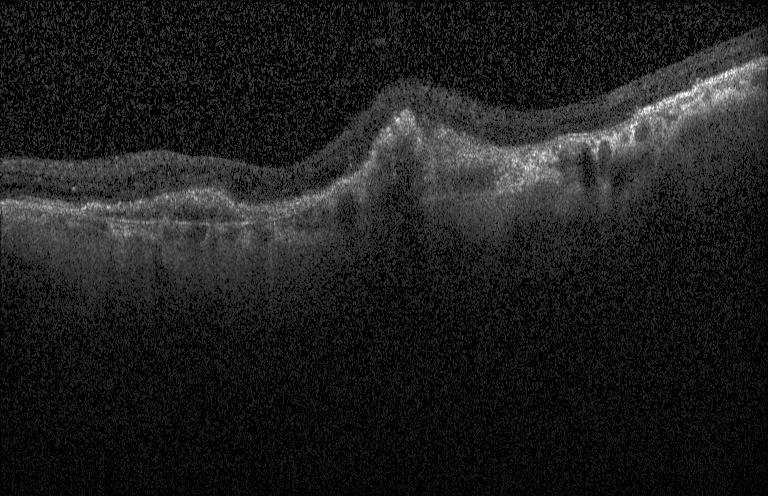 Optical coherence tomography scan.
Dx: a choroidal neovascular membrane.